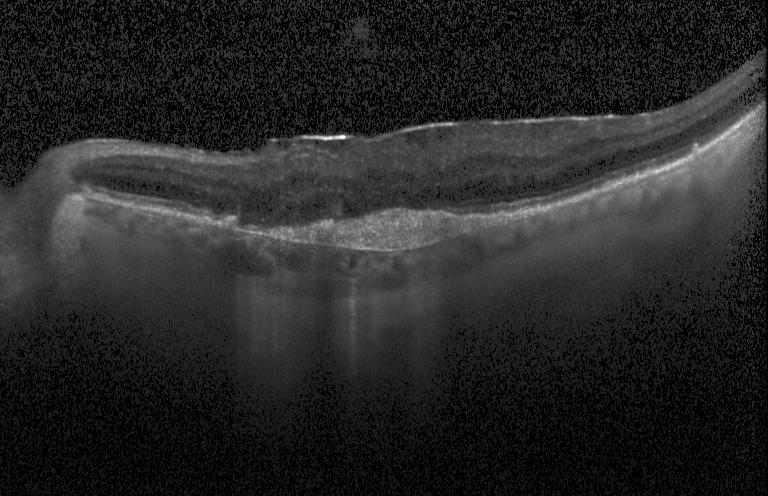 Diagnosis: choroidal neovascularization (CNV).